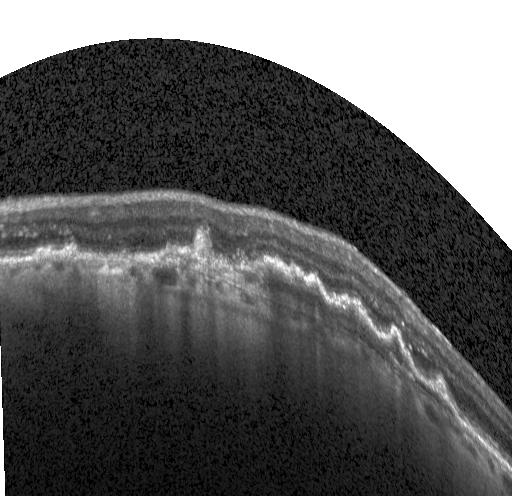
Spectral-domain optical coherence tomography · retinal OCT B-scan · fovea-centered.
Diagnosis: a choroidal neovascular membrane.